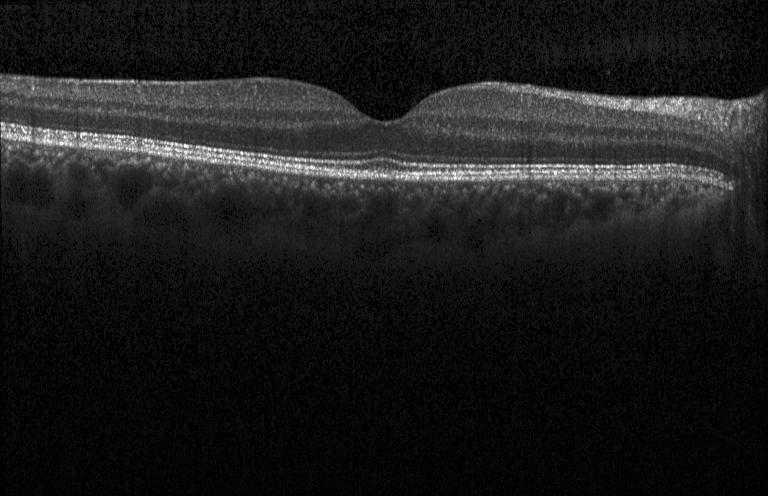
Spectral-domain OCT, retinal OCT cross-section, horizontal scan through the fovea — Assessment: no choroidal neovascularization, diabetic macular edema, or drusen.